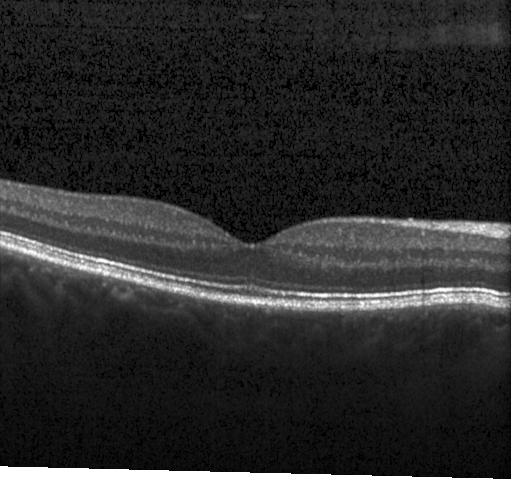

OCT finding: no choroidal neovascularization, no diabetic macular edema, and no drusen.